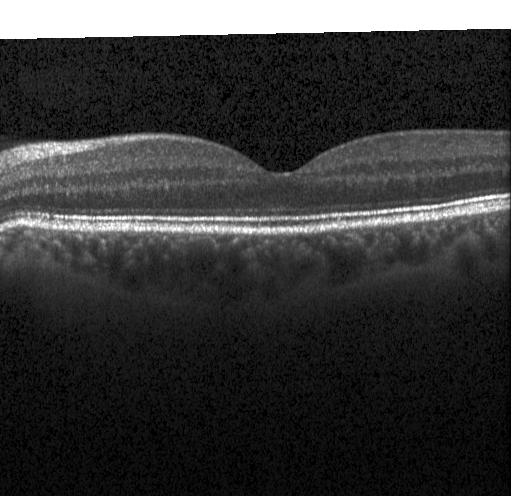

Diagnosis: no CNV, no DME, and no drusen.